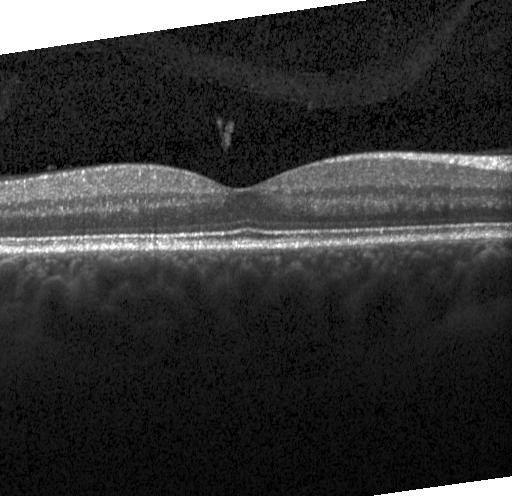
SD-OCT; horizontal scan through the fovea; optical coherence tomography B-scan. Finding: no choroidal neovascularization, diabetic macular edema, or drusen.